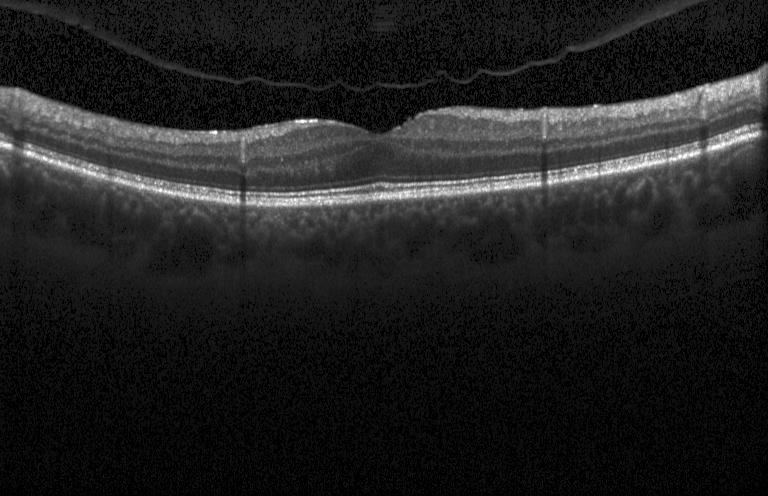
Acquired on a Heidelberg Spectralis · macular scan · optical coherence tomography B-scan
Diagnosis: neither choroidal neovascularization, diabetic macular edema, nor drusen.